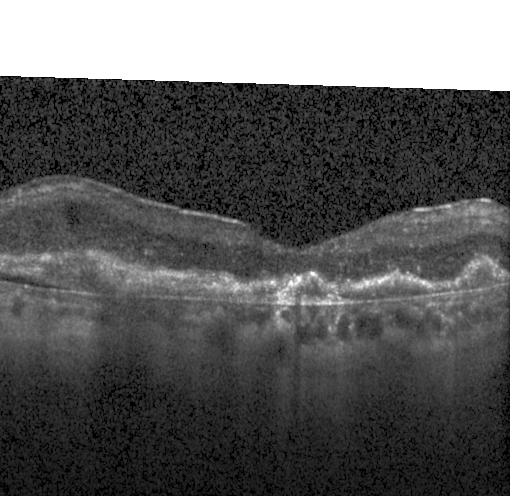

Centered on the fovea. Spectral-domain optical coherence tomography. Retinal OCT B-scan. Heidelberg Spectralis — Dx: choroidal neovascularization.